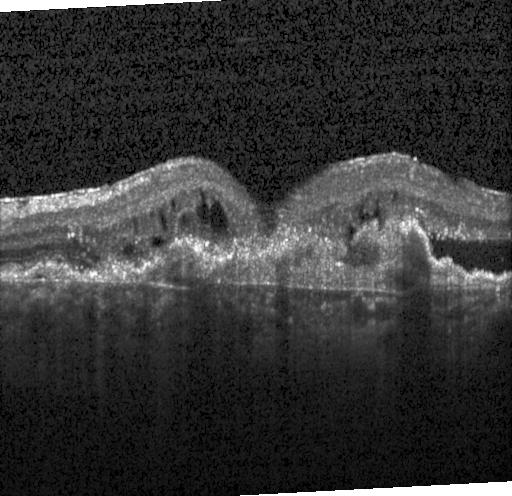 Impression: choroidal neovascularization.